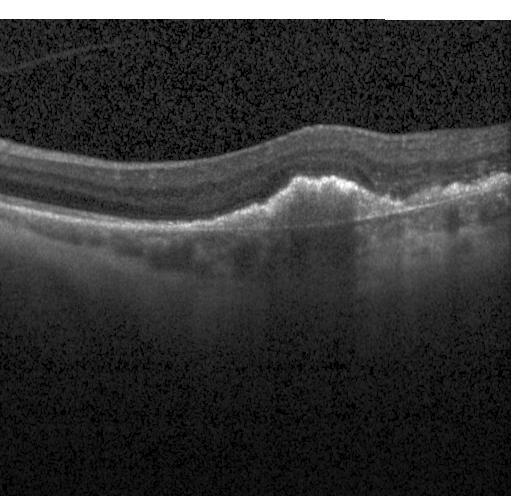 Macular OCT: a choroidal neovascular membrane.